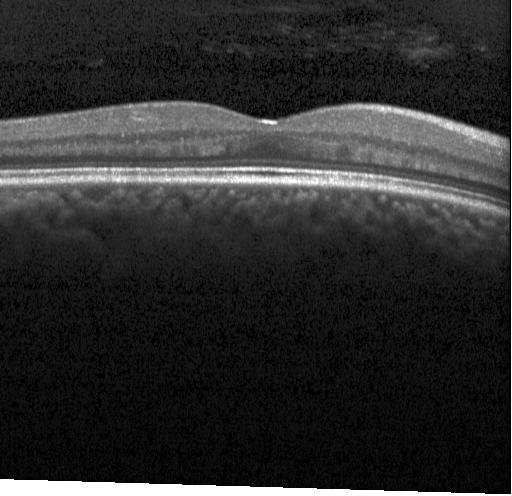
Heidelberg Spectralis, optical coherence tomography scan.
Neither choroidal neovascularization, diabetic macular edema, nor drusen.